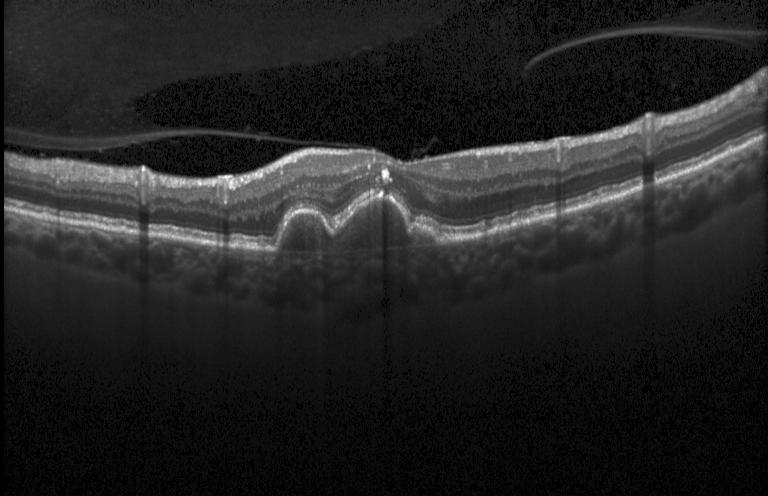 OCT finding: a choroidal neovascular membrane.